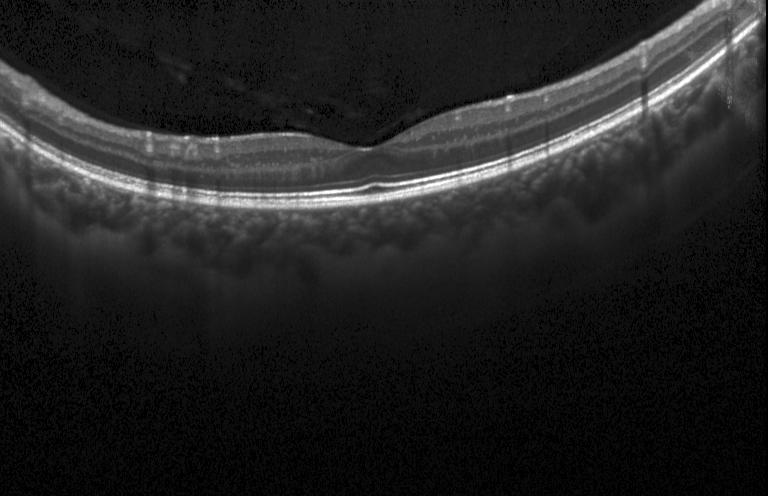

Retinal OCT cross-section · Heidelberg Spectralis · spectral-domain optical coherence tomography. Neither choroidal neovascularization, diabetic macular edema, nor drusen.